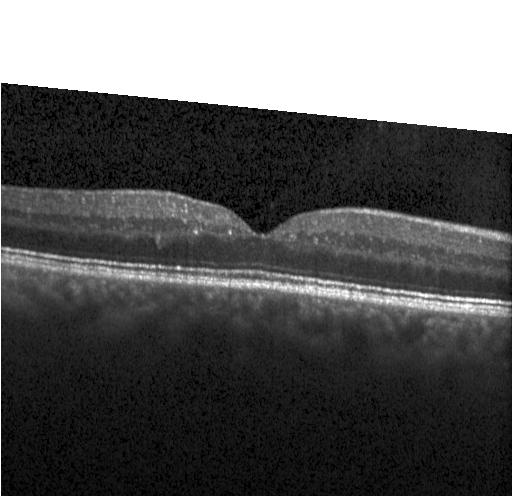 Optical coherence tomography B-scan · macular scan
Finding: neither CNV, DME, nor drusen.